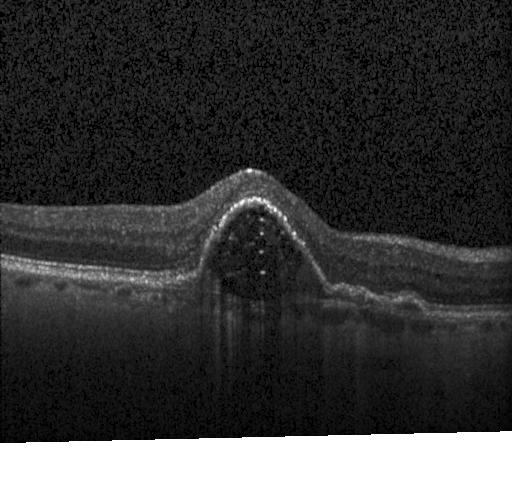 OCT B-scan; instrument: Heidelberg Spectralis
Diagnosis: choroidal neovascularization.